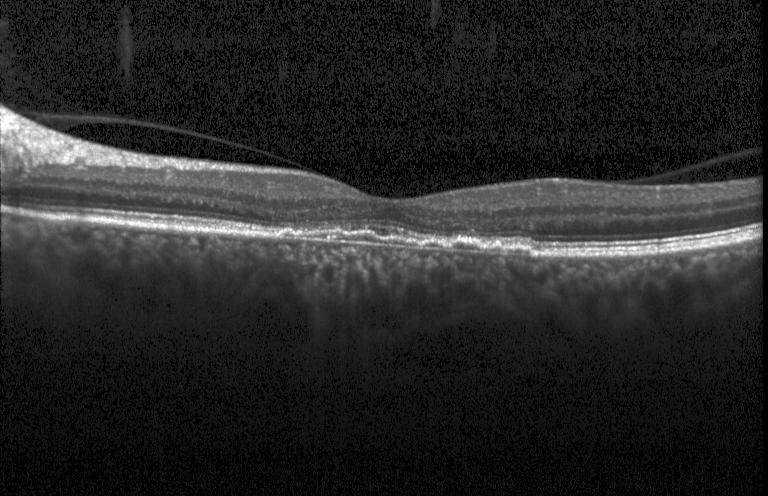 Instrument: Heidelberg Spectralis; spectral-domain OCT; optical coherence tomography scan; macular scan.
Finding: a choroidal neovascular membrane.